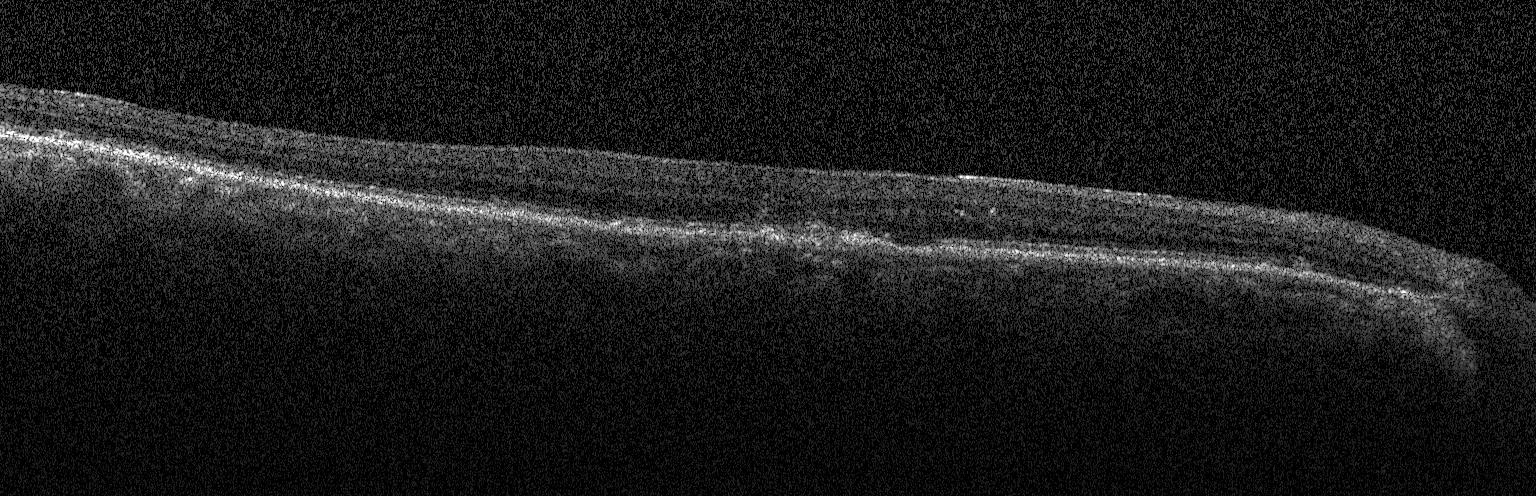 Acquired on a Heidelberg Spectralis. Spectral-domain OCT. Retinal OCT cross-section — The scan shows multiple drusen.